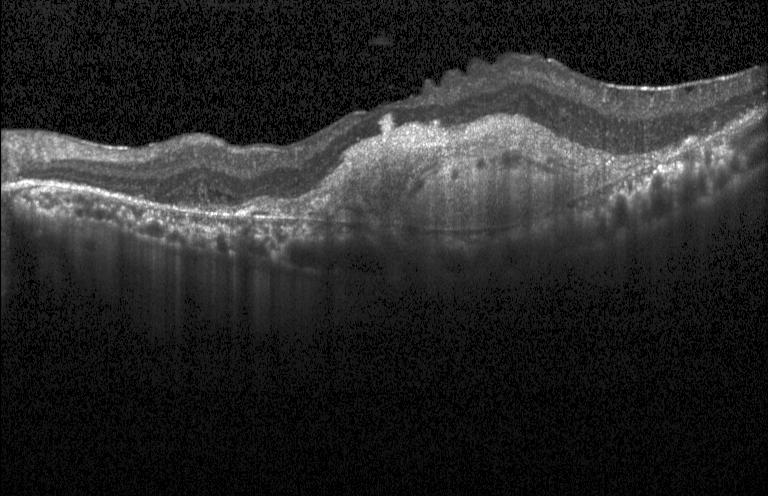
Spectral-domain OCT B-scan: CNV.